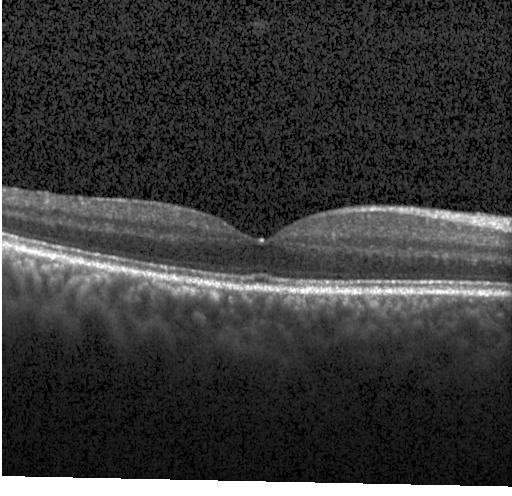

Retinal OCT B-scan.
The scan shows no choroidal neovascularization, no diabetic macular edema, and no drusen.